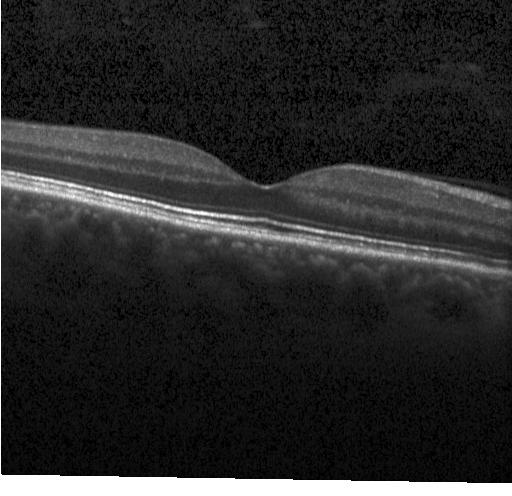 Finding: no evidence of choroidal neovascularization, diabetic macular edema, or drusen.